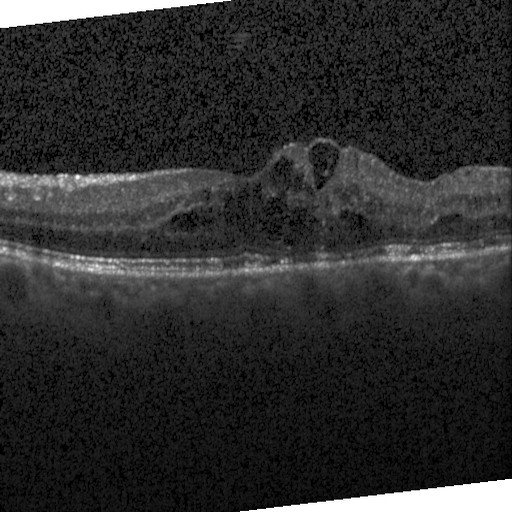

Optical coherence tomography scan
Diagnosis: diabetic macular edema.